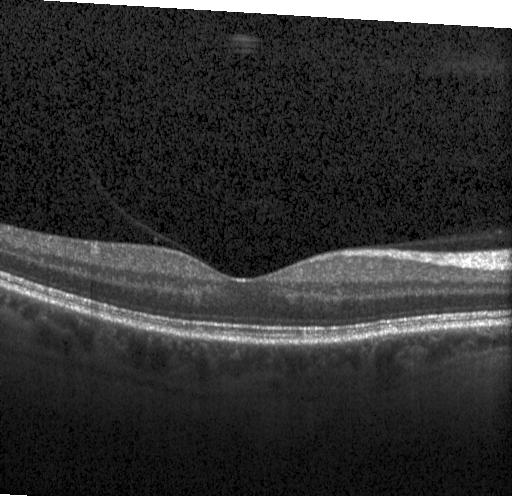 Spectral-domain optical coherence tomography. Heidelberg Spectralis. OCT B-scan. Centered on the fovea — Impression: no CNV, DME, or drusen.